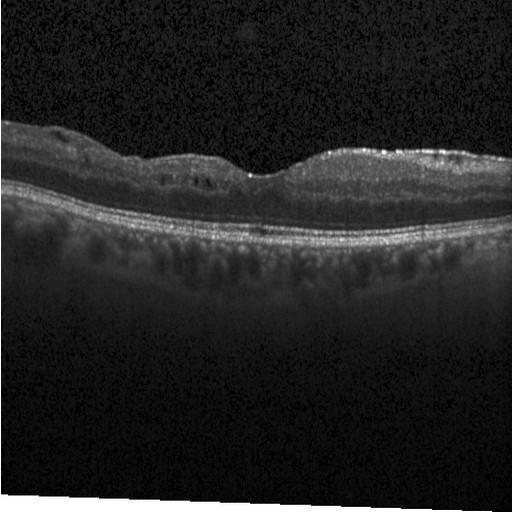 Optical coherence tomography scan · spectral-domain OCT.
Assessment: diabetic macular edema (DME).